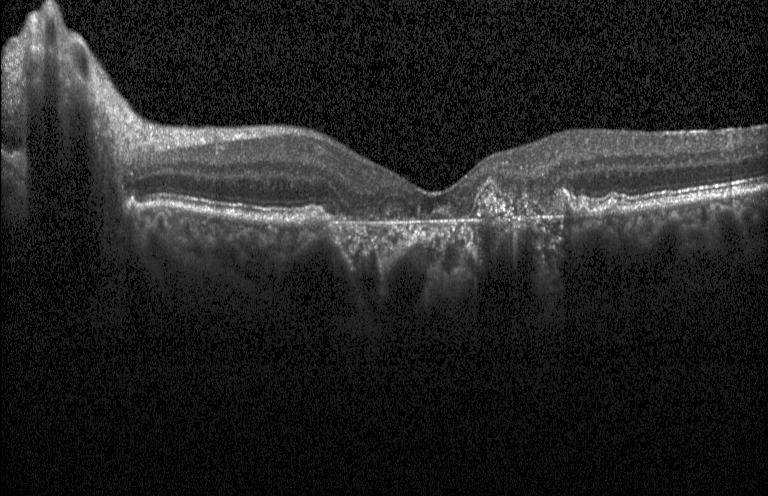 OCT B-scan. Horizontal scan through the fovea.
The scan shows choroidal neovascularization (CNV).